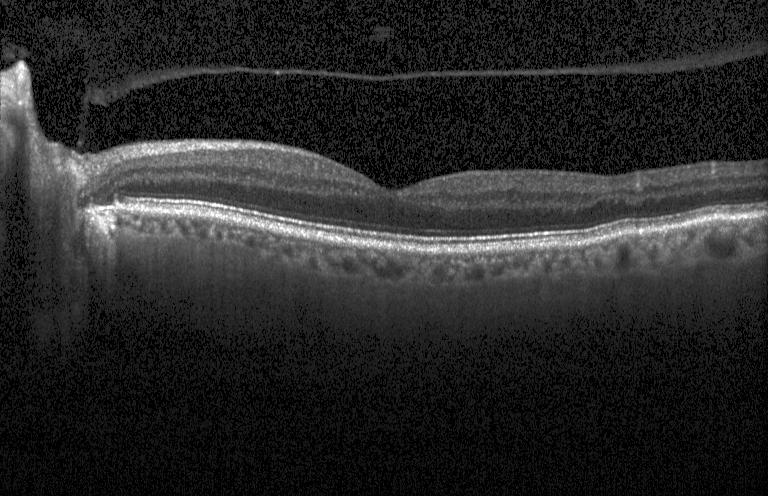

Optical coherence tomography scan — Assessment: neither choroidal neovascularization, diabetic macular edema, nor drusen.